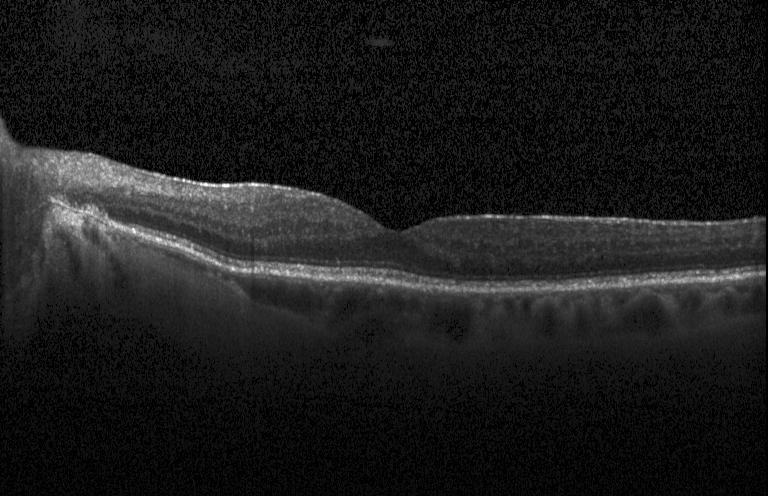 Macular scan, spectral-domain optical coherence tomography, optical coherence tomography scan
Finding: no evidence of choroidal neovascularization, diabetic macular edema, or drusen.